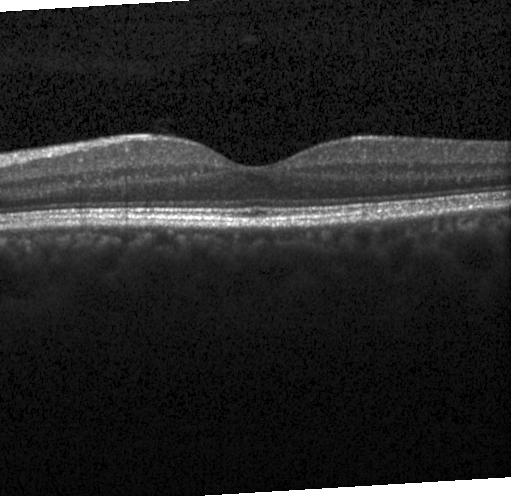
Finding: no evidence of choroidal neovascularization, diabetic macular edema, or drusen.